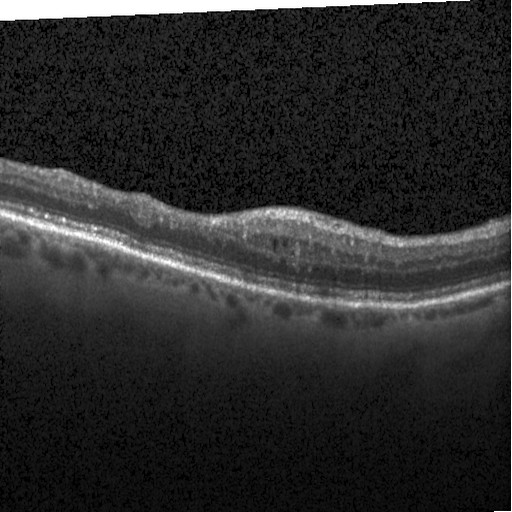 Heidelberg Spectralis · optical coherence tomography scan
This B-scan demonstrates diabetic macular edema.